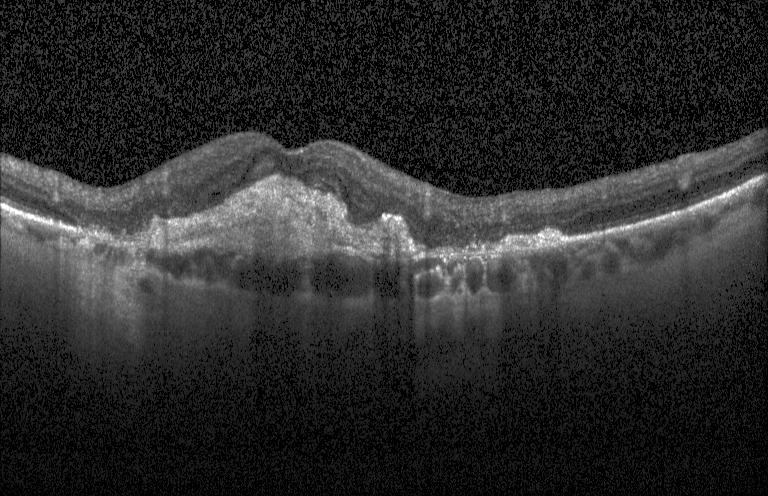 Finding: a choroidal neovascular membrane.